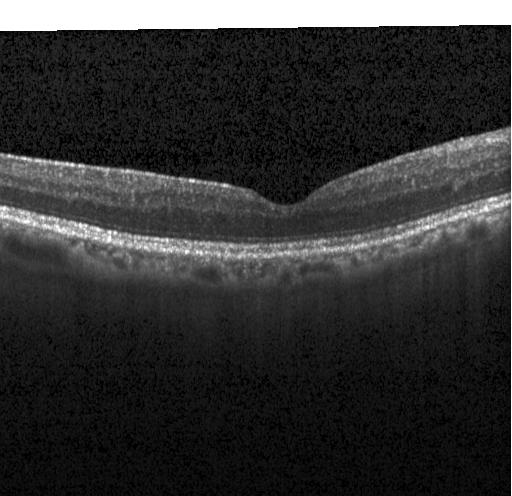 OCT finding: no choroidal neovascularization, no diabetic macular edema, and no drusen.